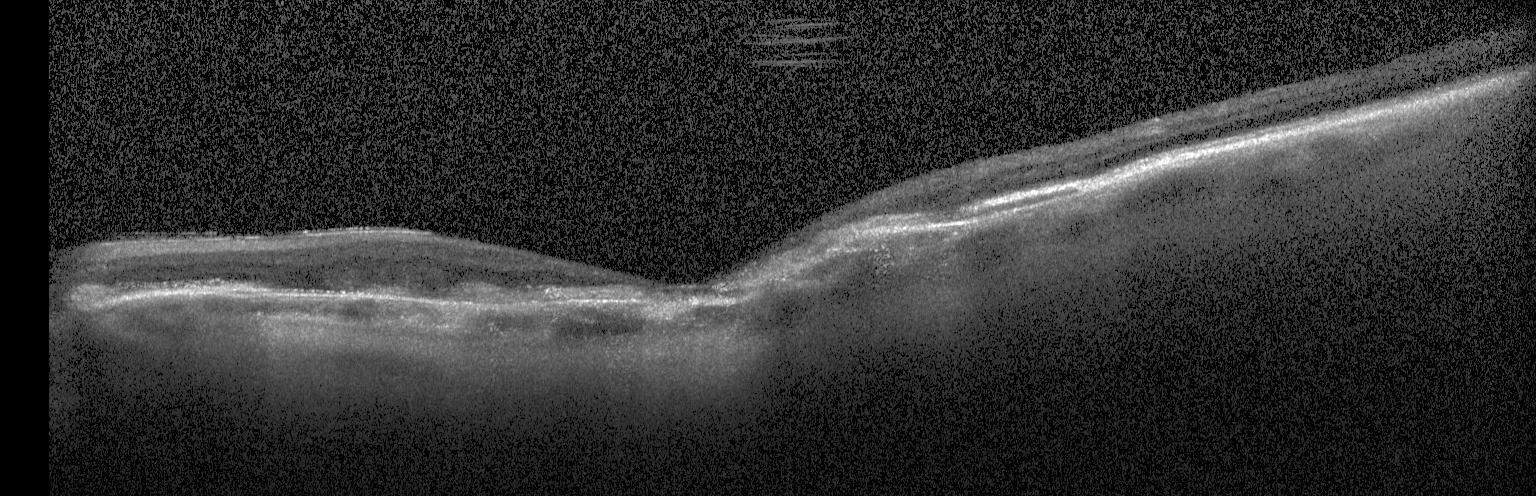 Impression: a choroidal neovascular membrane.